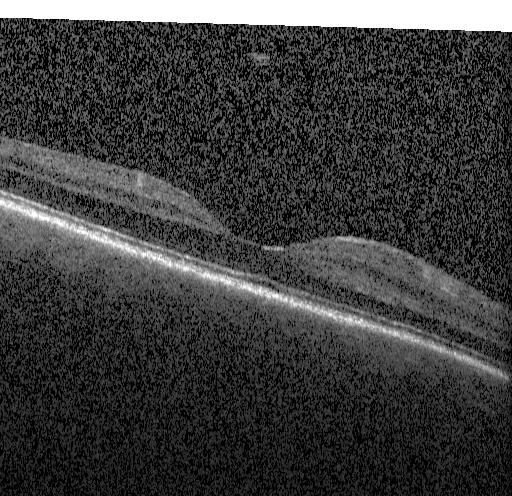
Spectral-domain OCT · OCT B-scan.
Assessment: no evidence of CNV, DME, or drusen.